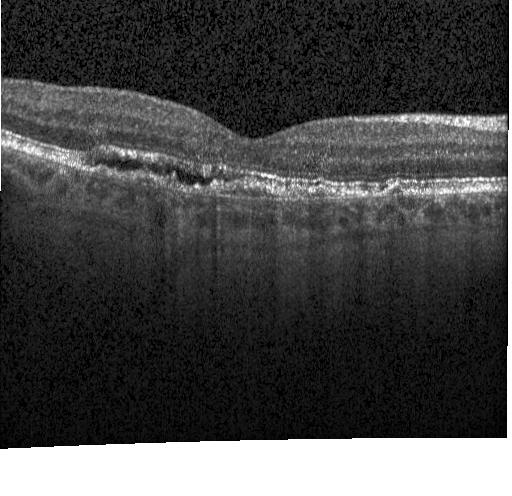
Macular OCT demonstrating a choroidal neovascular membrane.